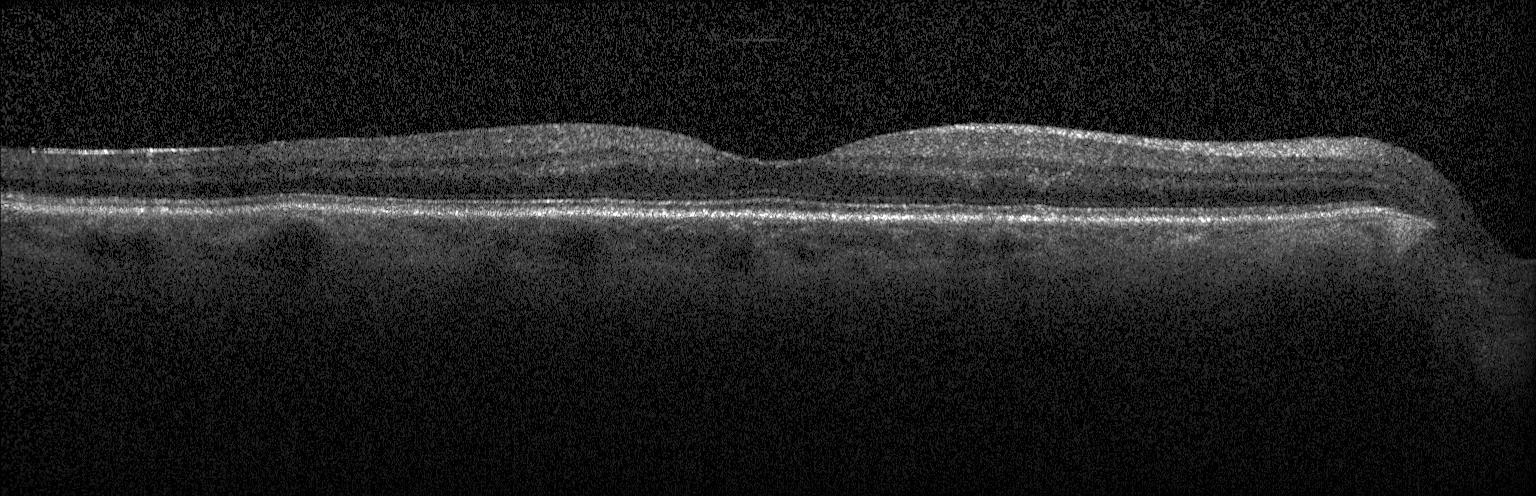 Acquired on a Heidelberg Spectralis · OCT line scan.
Impression: neither choroidal neovascularization, diabetic macular edema, nor drusen.